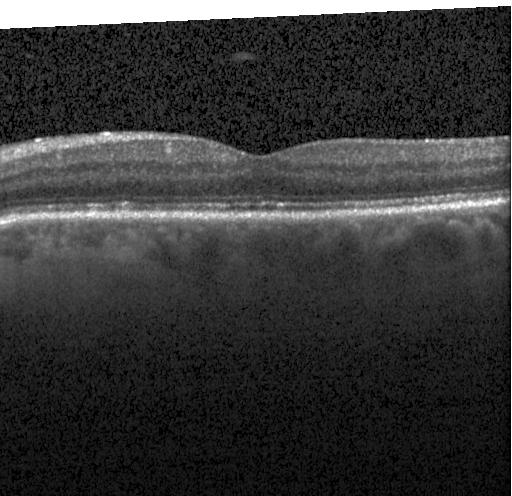
Through the macula · retinal OCT cross-section
OCT finding: no choroidal neovascularization, no diabetic macular edema, and no drusen.